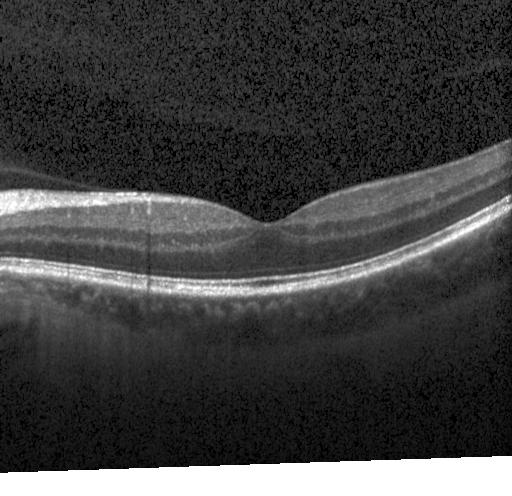

OCT line scan.
The scan shows no evidence of CNV, DME, or drusen.